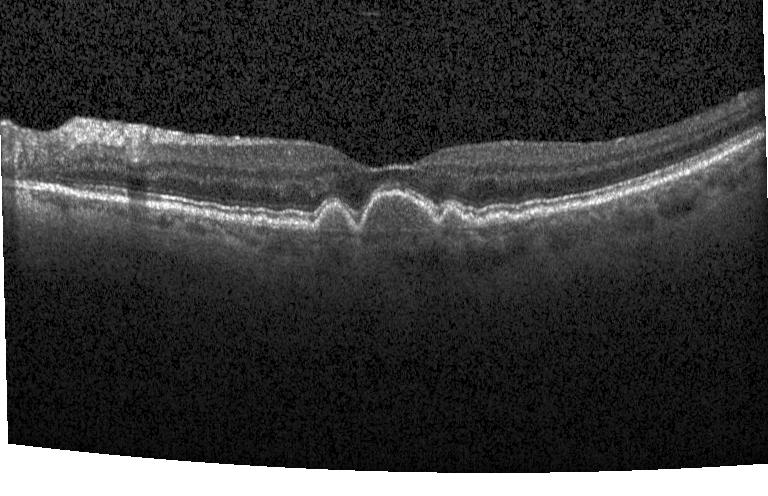

Assessment: multiple drusen.